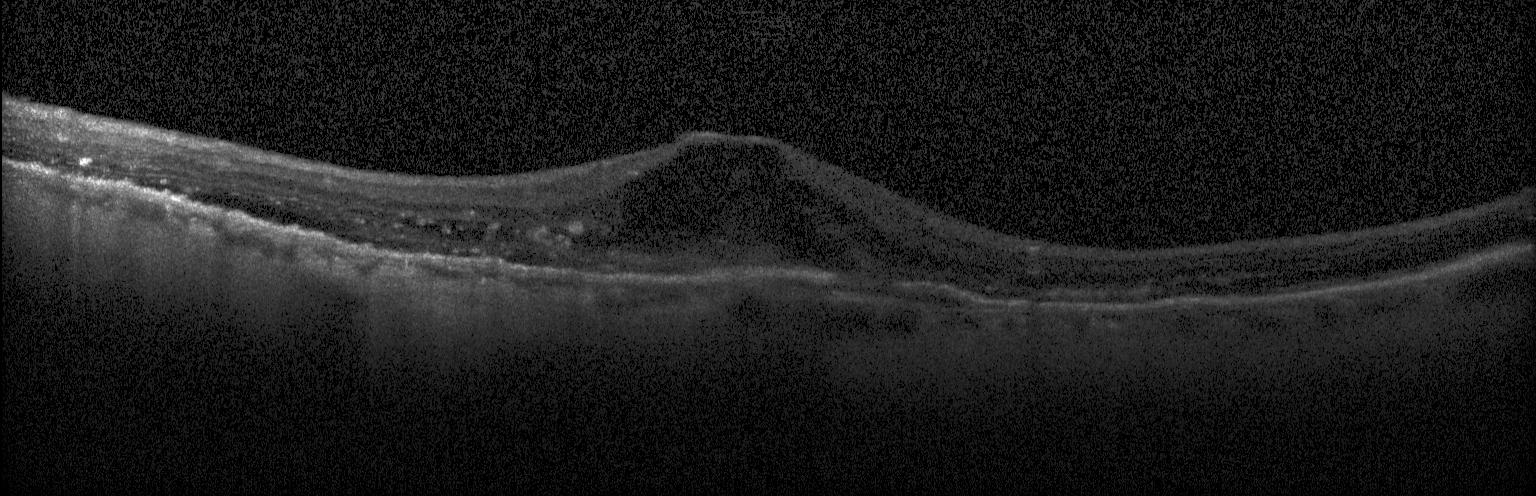 SD-OCT; retinal OCT B-scan — Choroidal neovascularization.